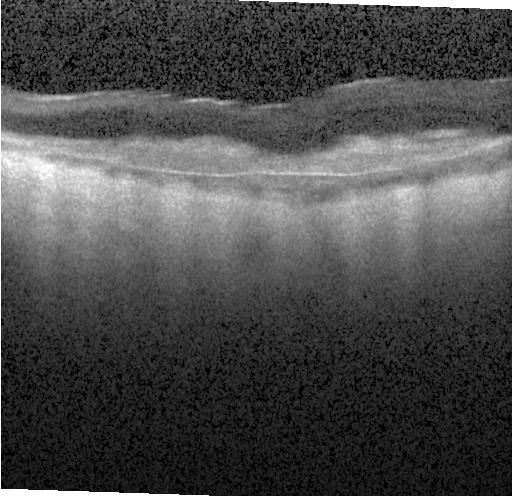
OCT line scan.
Diagnosis: a choroidal neovascular membrane.